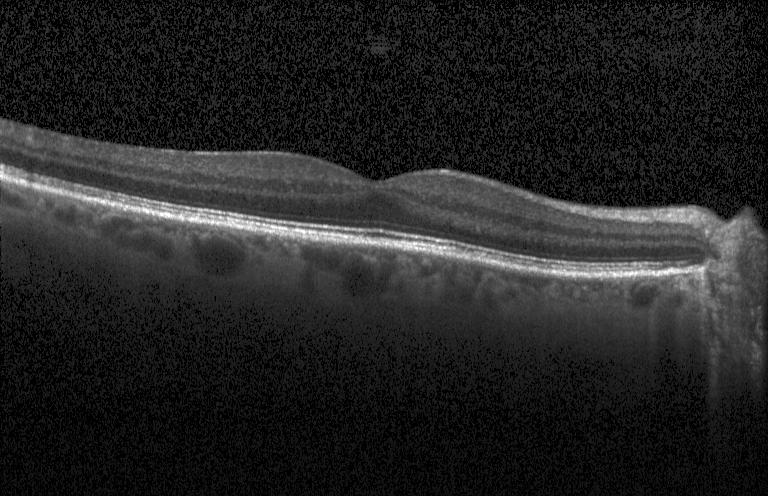
Instrument: Heidelberg Spectralis. Through the macula. Optical coherence tomography scan
Dx: no choroidal neovascularization, no diabetic macular edema, and no drusen.